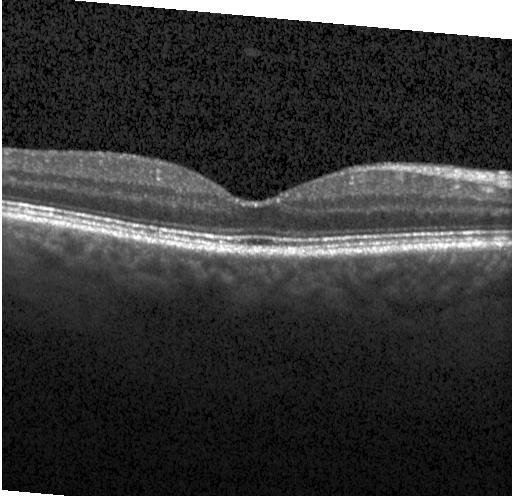

Heidelberg Spectralis · OCT B-scan · spectral-domain OCT.
Impression: no CNV, no DME, and no drusen.